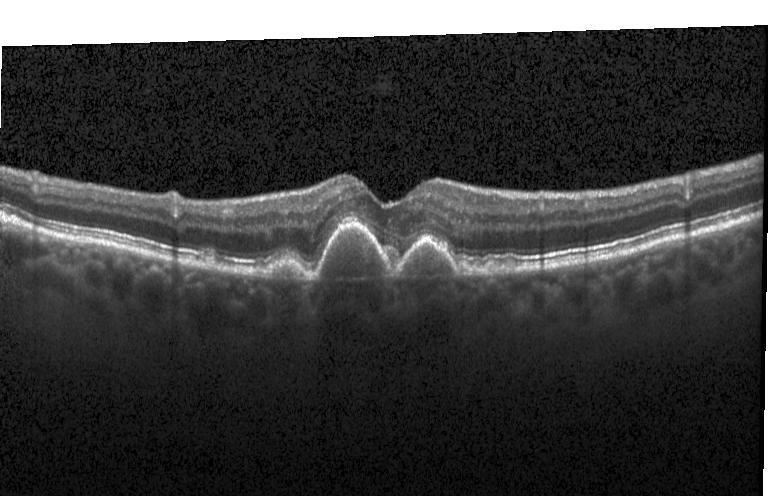 OCT finding: CNV.